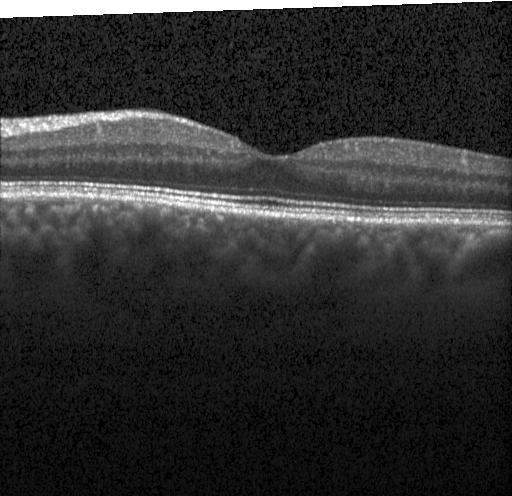 Macular scan; spectral-domain optical coherence tomography; retinal OCT B-scan; instrument: Heidelberg Spectralis
Macular OCT: no choroidal neovascularization, no diabetic macular edema, and no drusen.